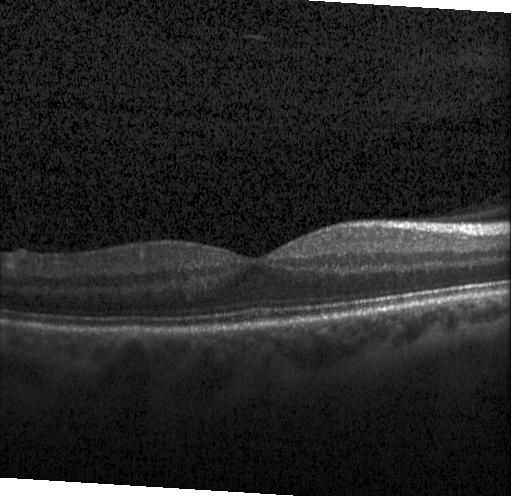 Optical coherence tomography scan
Impression: no choroidal neovascularization, no diabetic macular edema, and no drusen.